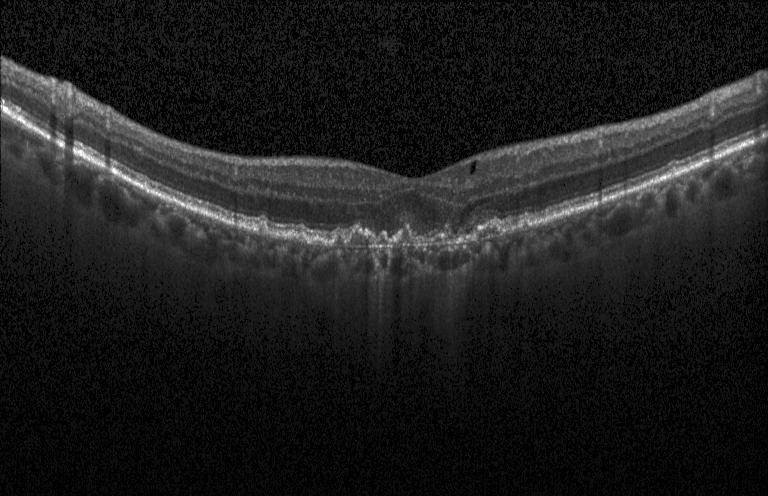
Macular OCT demonstrating choroidal neovascularization.